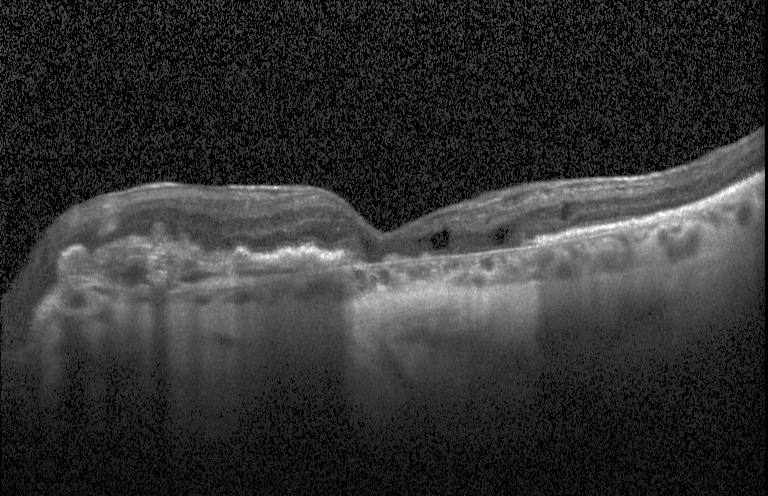

Retinal OCT B-scan.
A choroidal neovascular membrane.